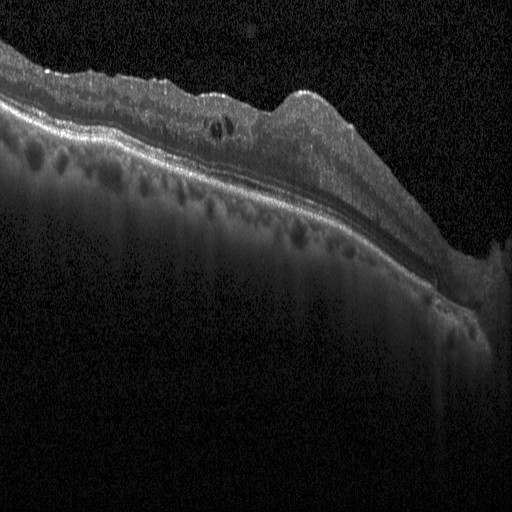
Retinal OCT B-scan, centered on the fovea. Diabetic macular edema (DME).